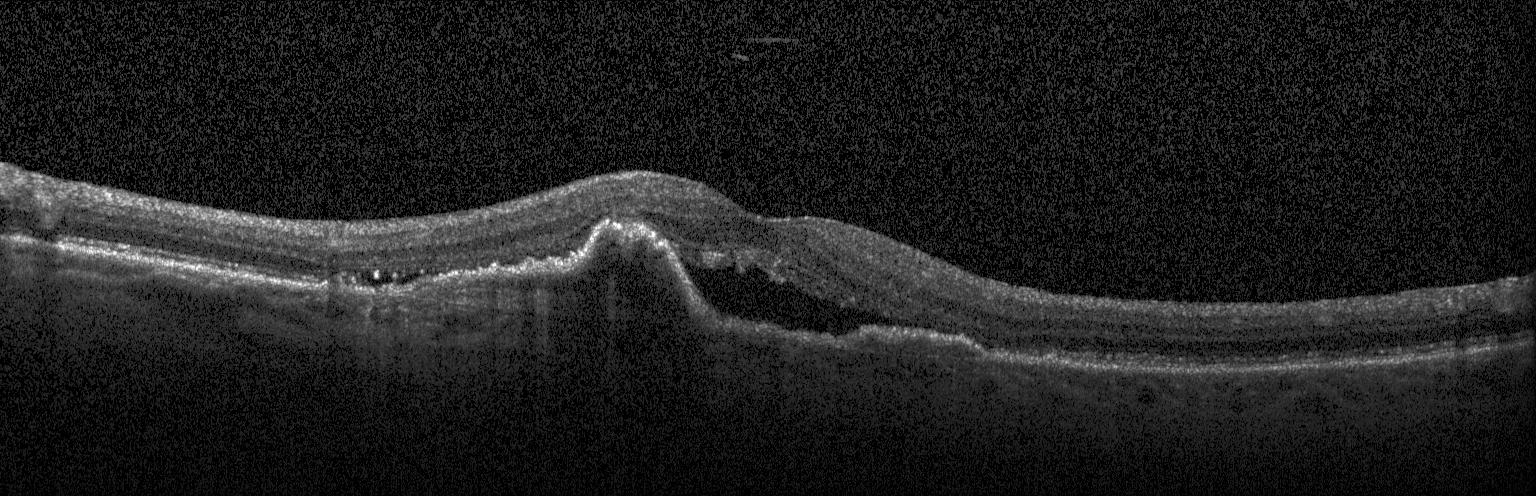
OCT finding: choroidal neovascularization.